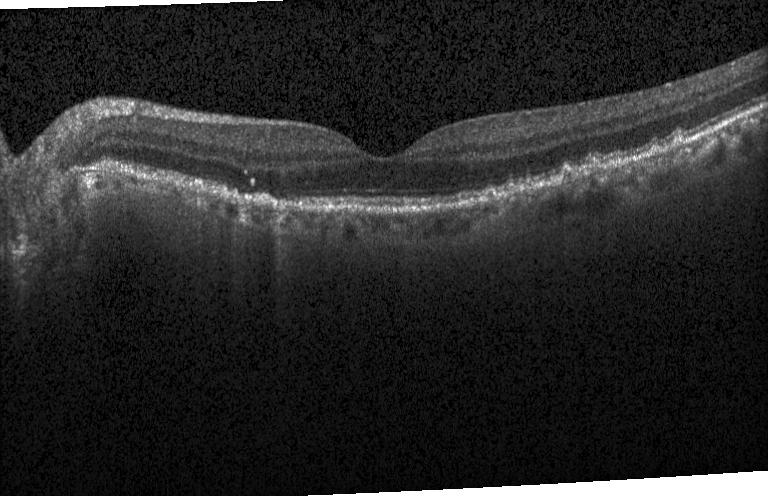
Diagnosis: multiple drusen.